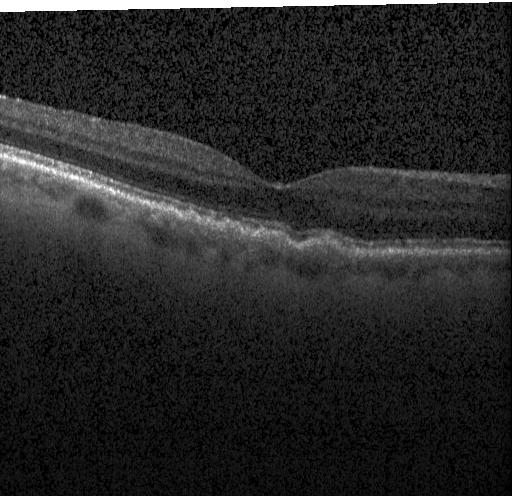
Macular OCT: multiple drusen.